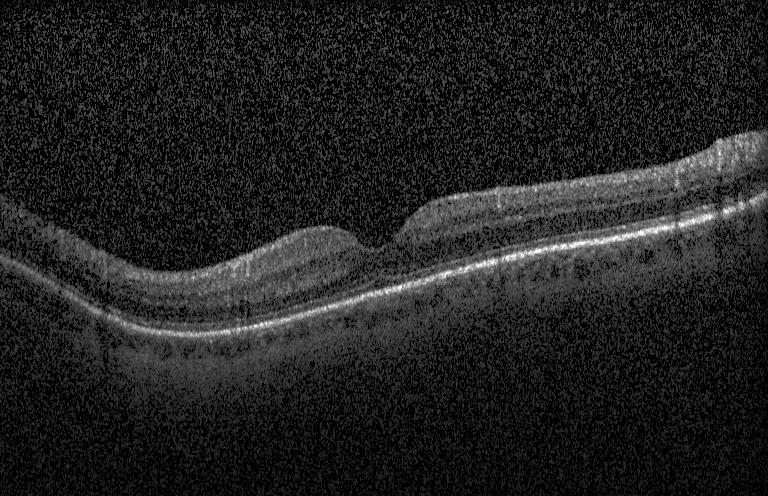 Retinal OCT cross-section showing neither choroidal neovascularization, diabetic macular edema, nor drusen.